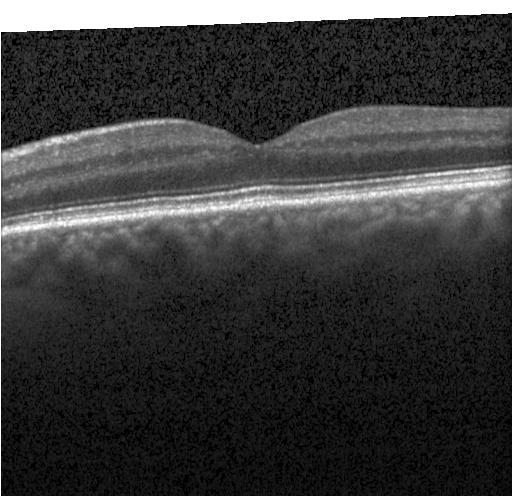

Optical coherence tomography scan. Assessment: no choroidal neovascularization, no diabetic macular edema, and no drusen.